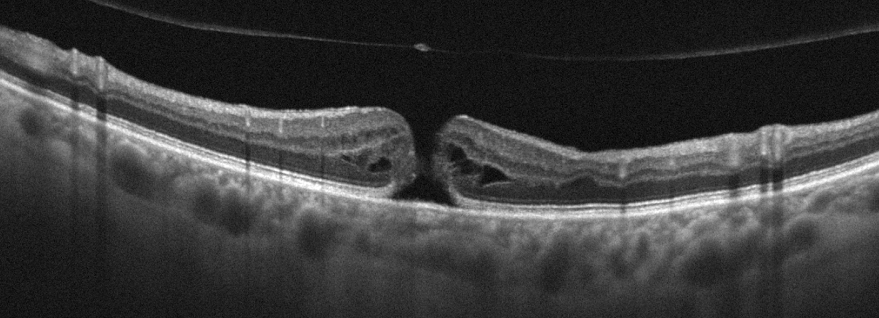
Optical coherence tomography scan, macular scan — Macular OCT: VID.